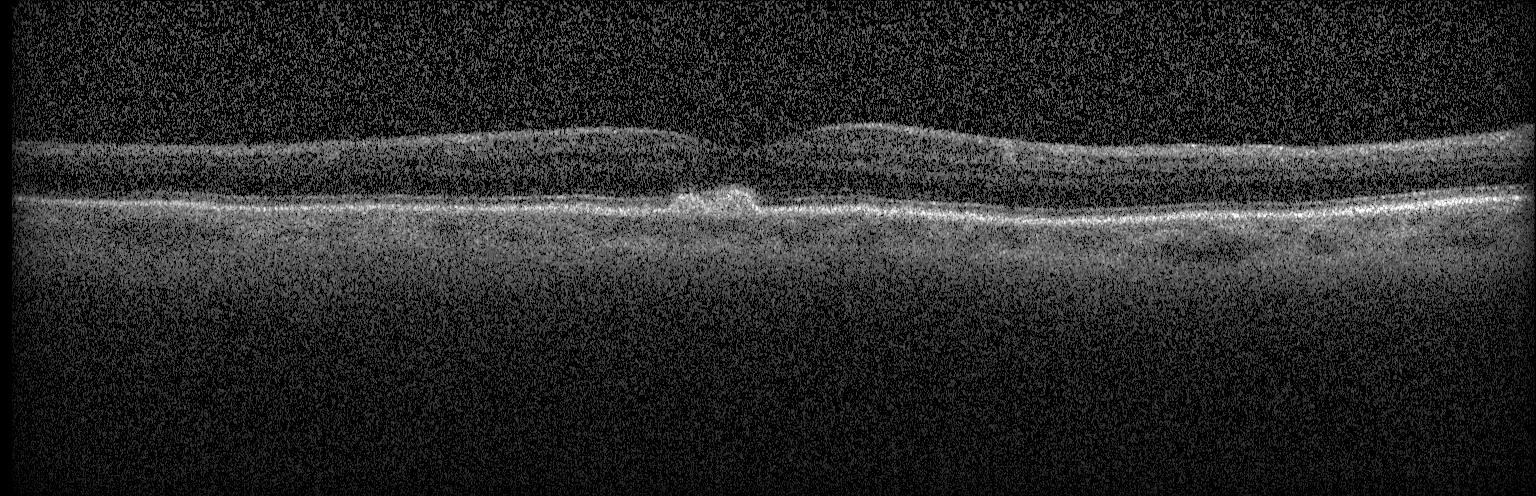
Optical coherence tomography scan. Dx: drusen.